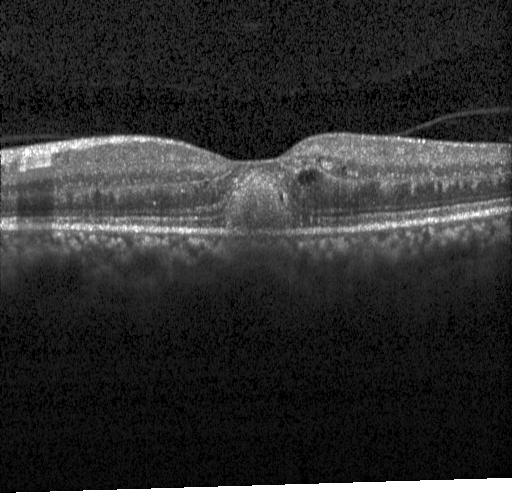 Centered on the fovea; acquired on a Heidelberg Spectralis; optical coherence tomography scan; spectral-domain OCT.
This B-scan demonstrates CNV.